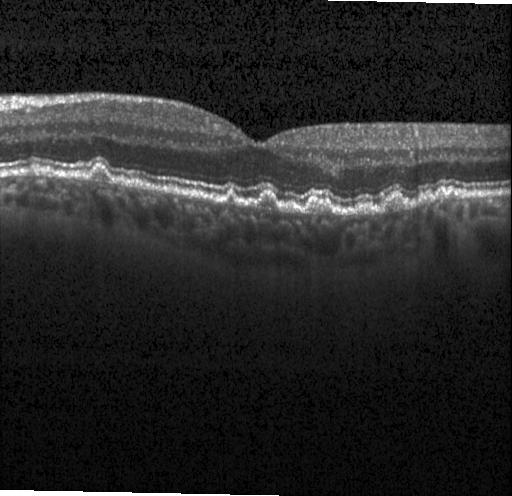
Retinal OCT cross-section showing sub-RPE drusenoid deposits.